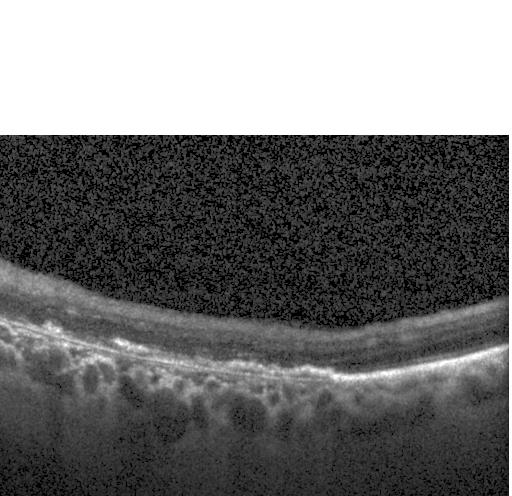

OCT finding: a choroidal neovascular membrane.